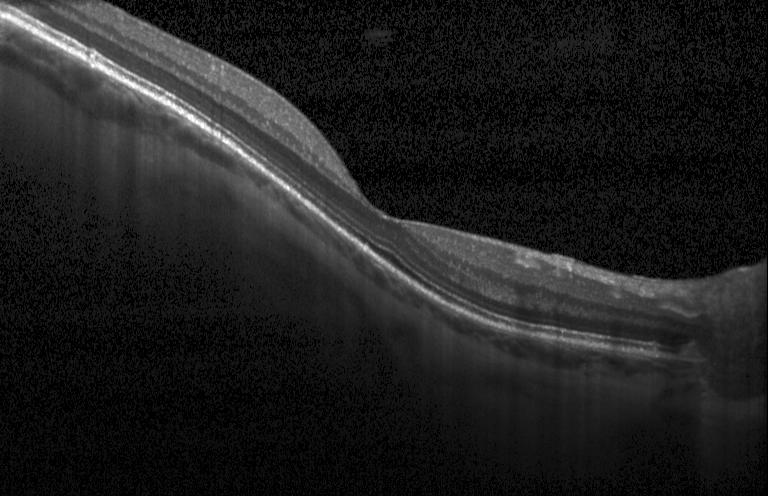
Impression: no CNV, no DME, and no drusen.